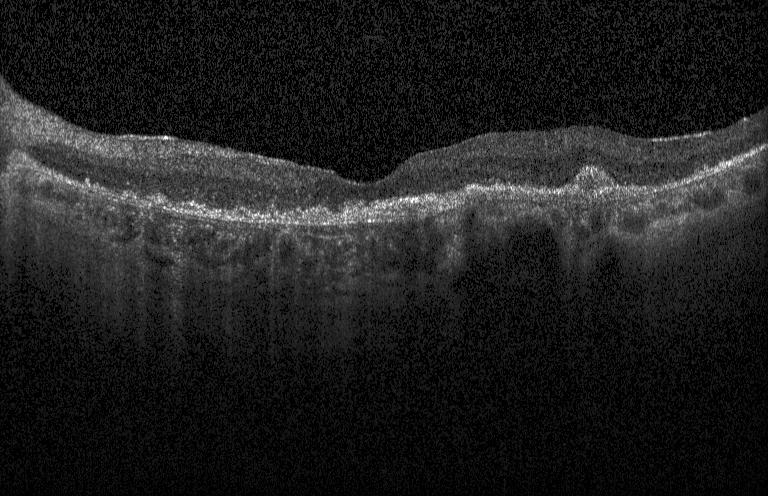 Spectral-domain optical coherence tomography · acquired on a Heidelberg Spectralis · centered on the fovea · retinal OCT cross-section
Impression: a choroidal neovascular membrane.